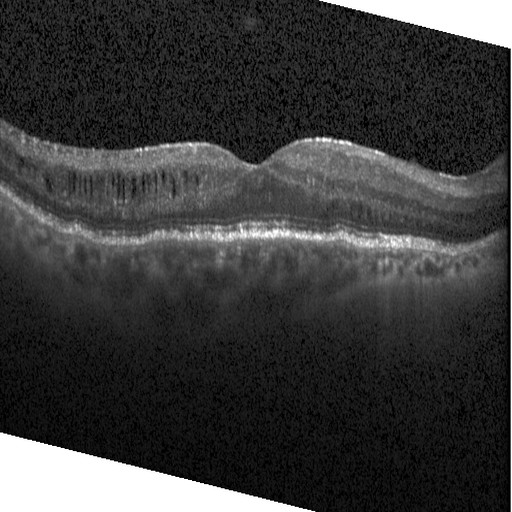
Diagnosis: DME.